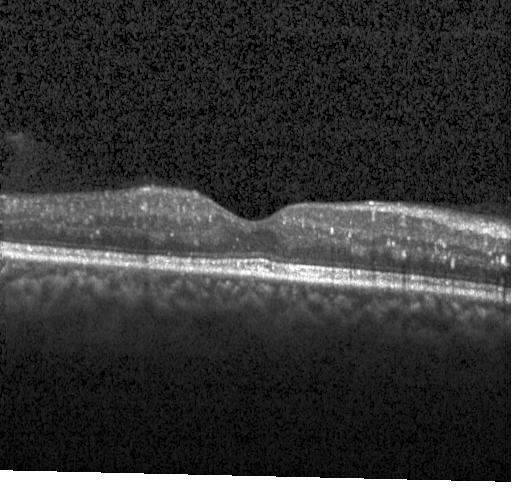 Retinal OCT cross-section. Impression: diabetic macular edema (DME).